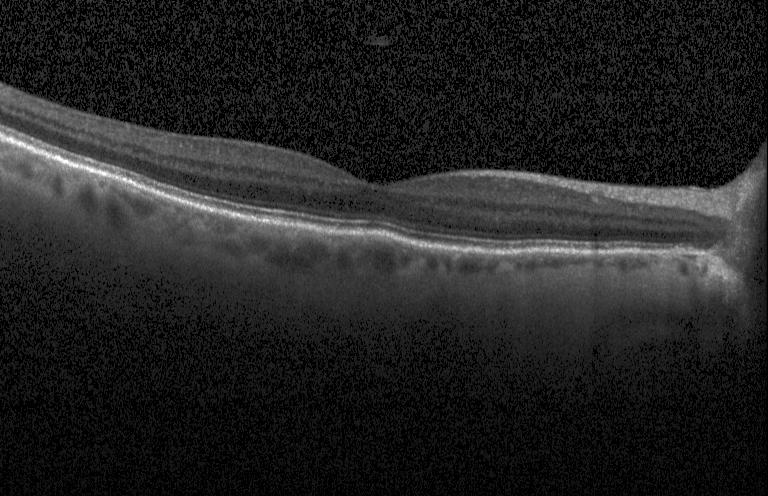 Retinal OCT cross-section.
Macular OCT: neither CNV, DME, nor drusen.